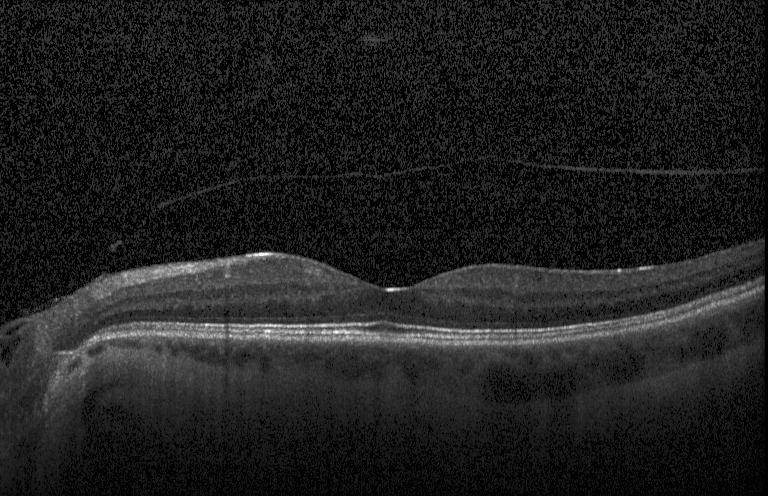 OCT line scan; instrument: Heidelberg Spectralis; macular scan. Finding: no choroidal neovascularization, no diabetic macular edema, and no drusen.